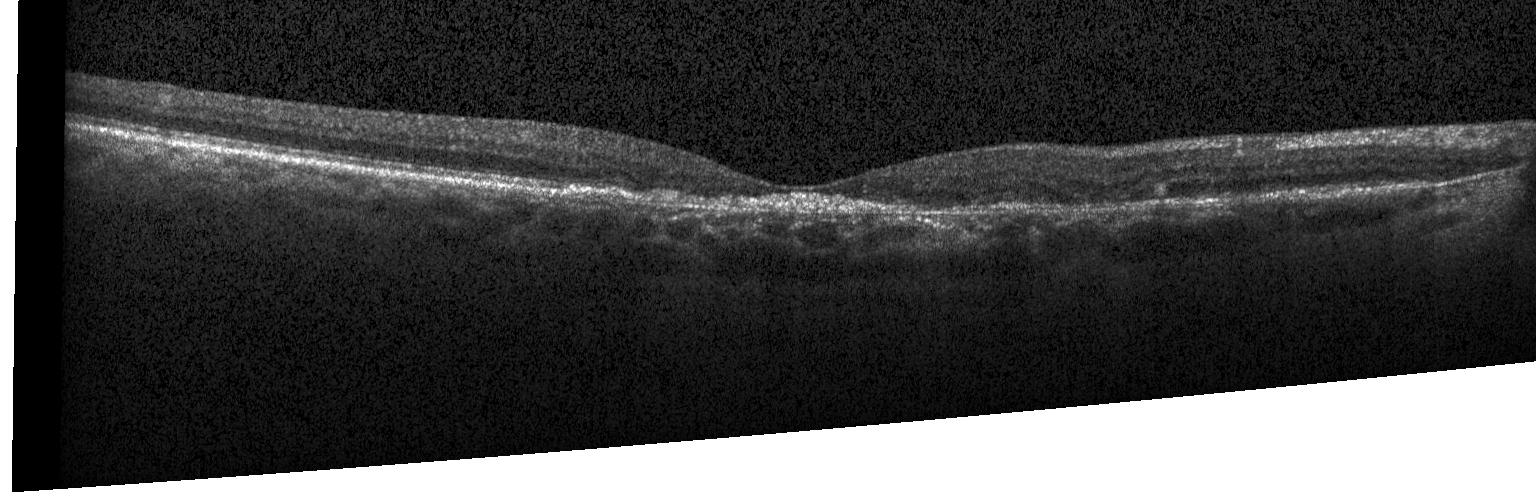
Macular OCT demonstrating choroidal neovascularization.